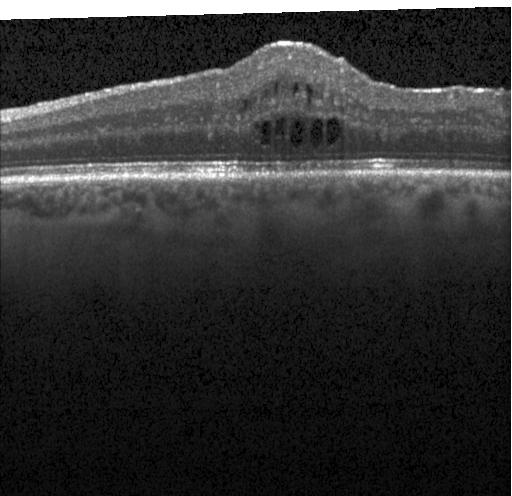 Impression: diabetic macular edema (DME).